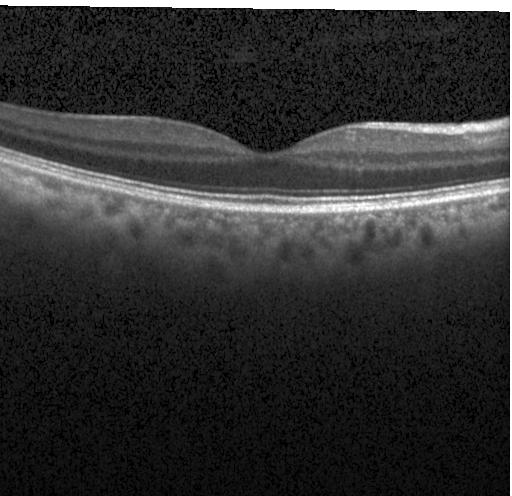

OCT line scan.
Diagnosis: no CNV, DME, or drusen.